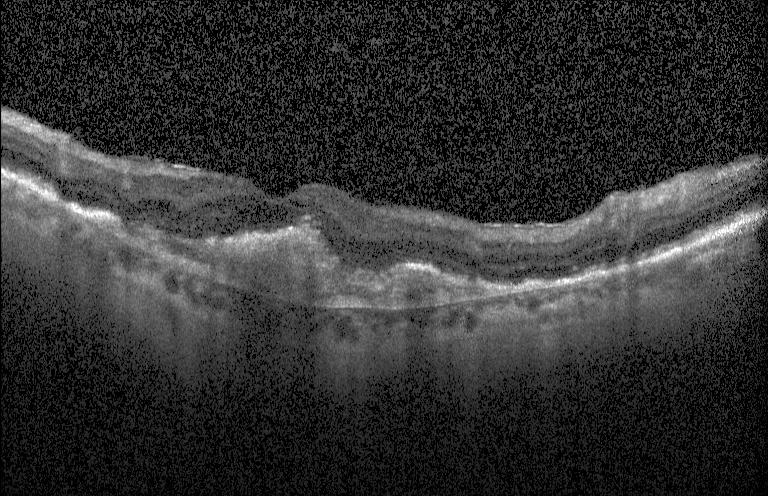 OCT scan showing choroidal neovascularization (CNV).